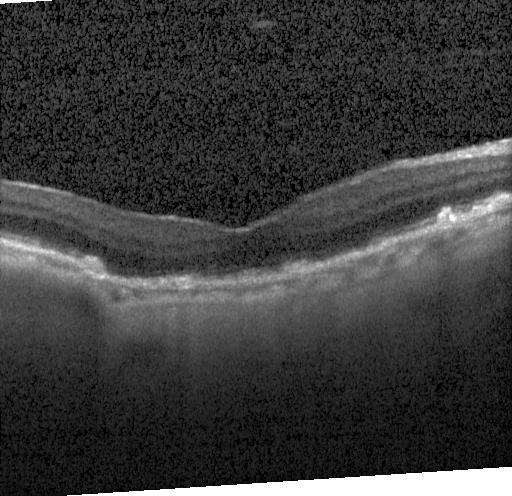 Horizontal scan through the fovea, optical coherence tomography scan, Heidelberg Spectralis OCT system.
Impression: choroidal neovascularization (CNV).